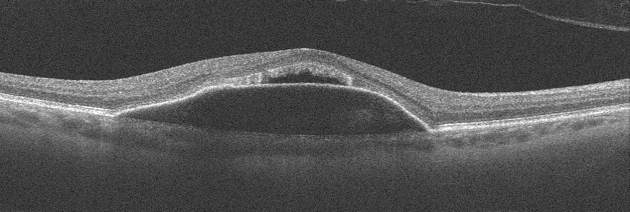 Optovue Avanti RTVue XR. Through the macula. Optical coherence tomography scan. Oculus dexter — Age-related macular degeneration.